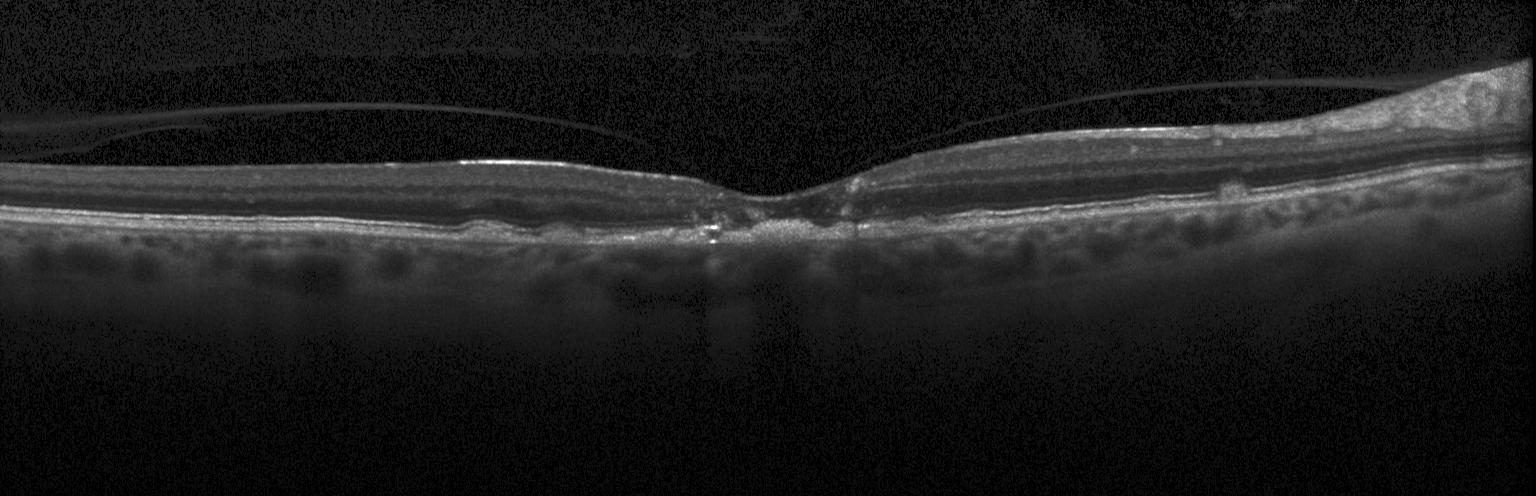 OCT B-scan. Assessment: choroidal neovascularization.